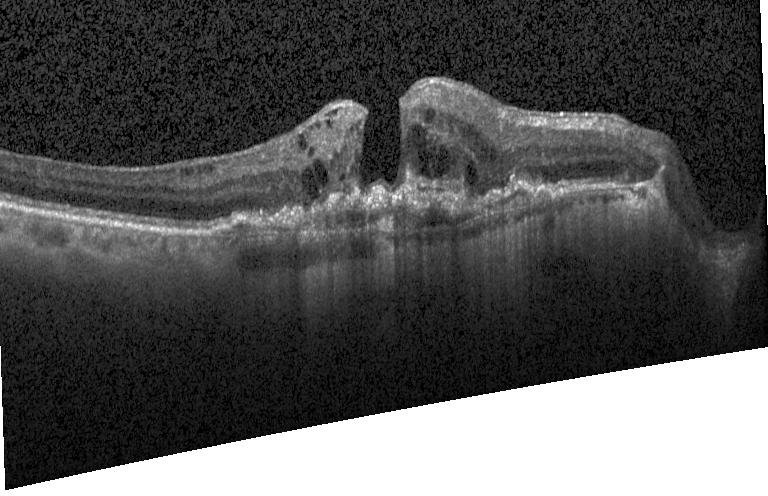 Centered on the fovea. Spectral-domain OCT. OCT line scan. This B-scan demonstrates a choroidal neovascular membrane.